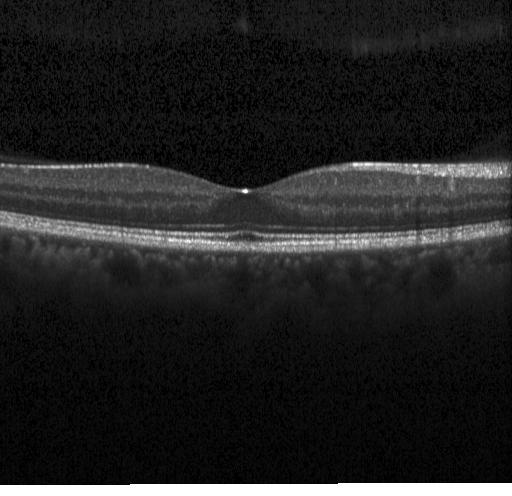

Acquired on a Heidelberg Spectralis; spectral-domain optical coherence tomography; through the macula; retinal OCT B-scan.
Assessment: no choroidal neovascularization, no diabetic macular edema, and no drusen.